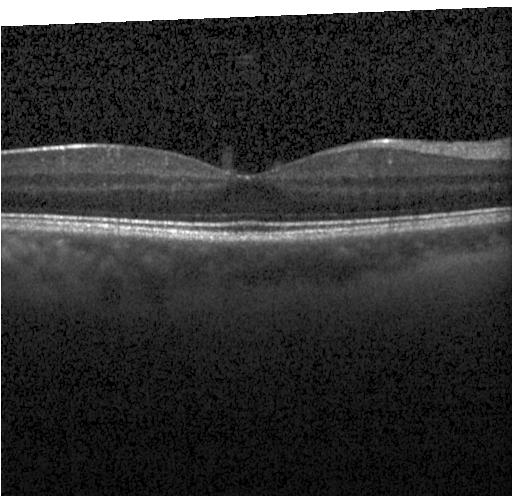
Impression: no CNV, no DME, and no drusen.